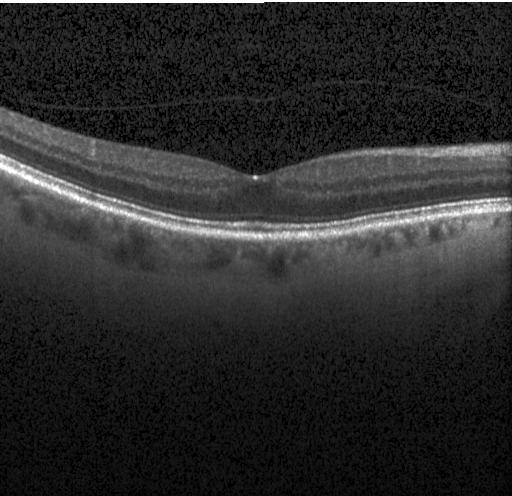
OCT line scan. SD-OCT. Fovea-centered. Heidelberg Spectralis OCT system.
Dx: no evidence of choroidal neovascularization, diabetic macular edema, or drusen.